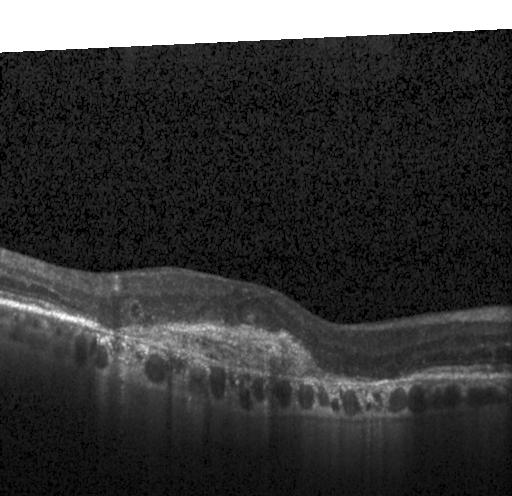 Through the macula; Heidelberg Spectralis OCT system; SD-OCT; optical coherence tomography B-scan. A choroidal neovascular membrane.